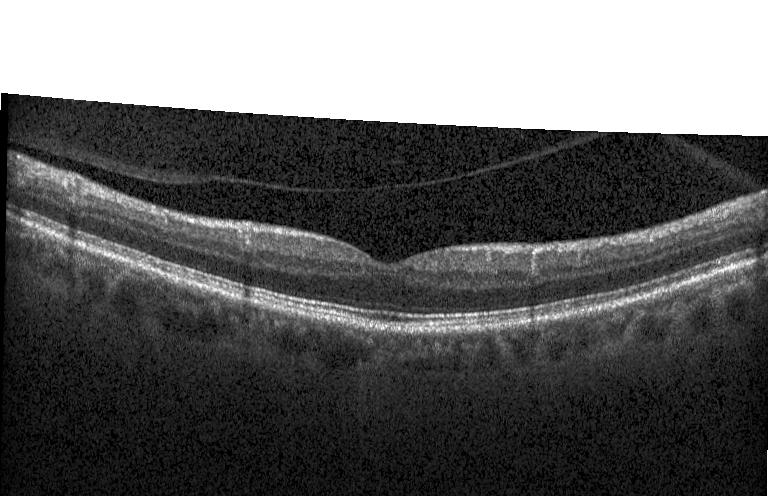
Assessment: no choroidal neovascularization, no diabetic macular edema, and no drusen.